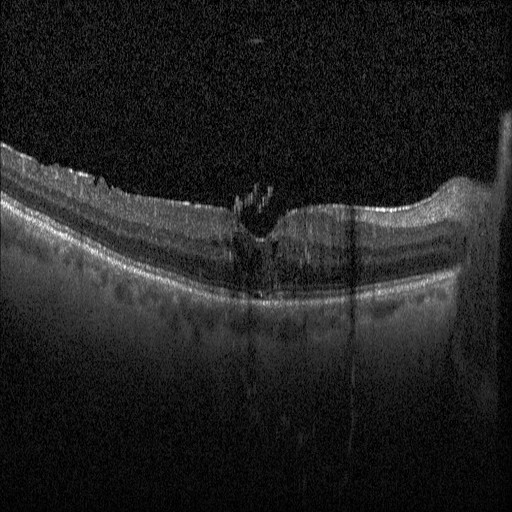
Retinal OCT B-scan
Macular OCT: diabetic macular edema (DME).